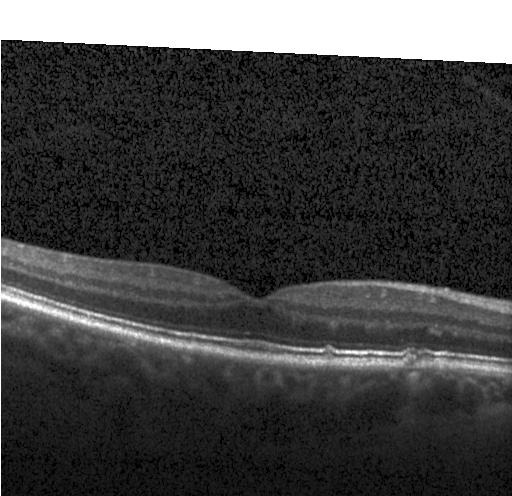 Impression: drusen.